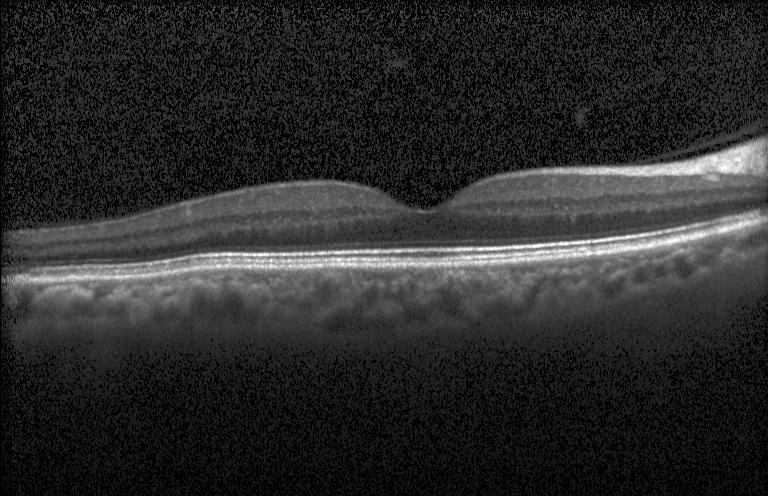

Optical coherence tomography scan · spectral-domain OCT · horizontal scan through the fovea · instrument: Heidelberg Spectralis.
This B-scan demonstrates no choroidal neovascularization, no diabetic macular edema, and no drusen.